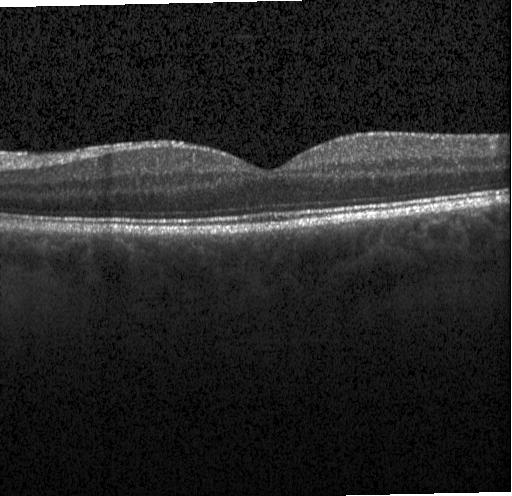 Diagnosis: no evidence of CNV, DME, or drusen.